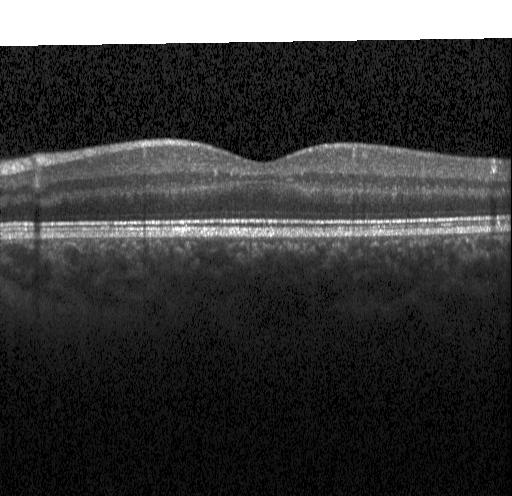 OCT line scan.
OCT finding: no evidence of CNV, DME, or drusen.